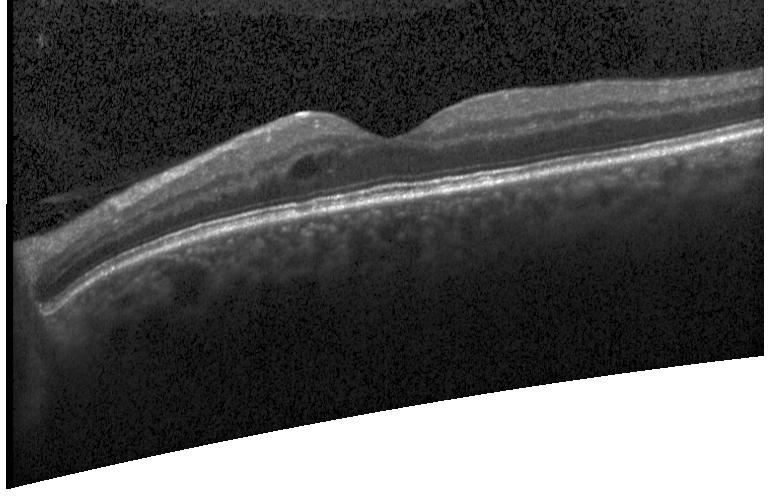

Spectral-domain optical coherence tomography; retinal OCT B-scan. Impression: diabetic macular edema.